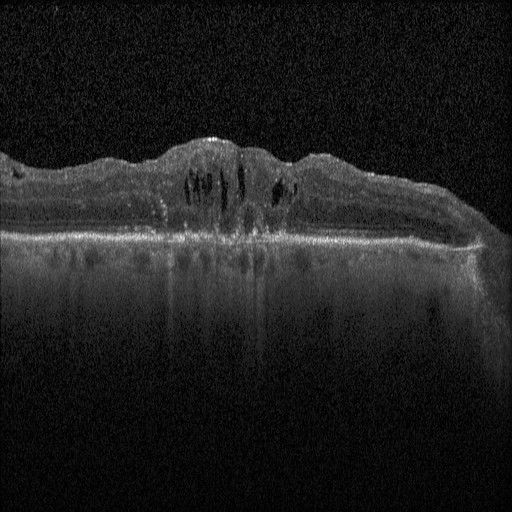 Spectral-domain optical coherence tomography; OCT B-scan; horizontal scan through the fovea — The scan shows diabetic macular edema.